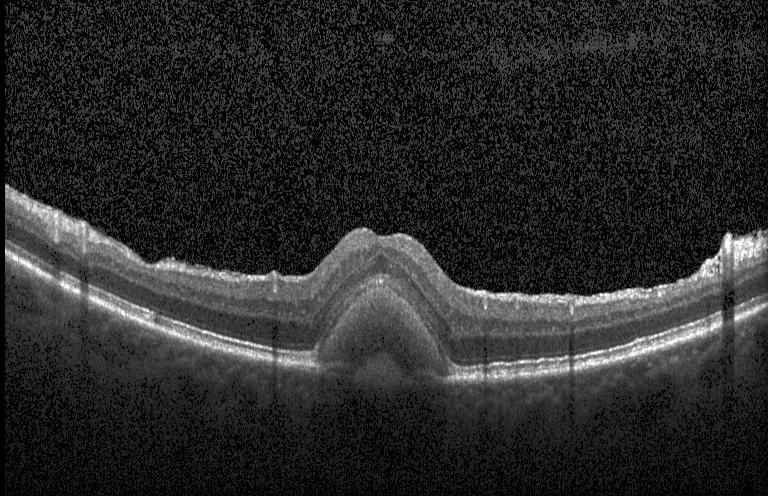

Finding: a choroidal neovascular membrane.